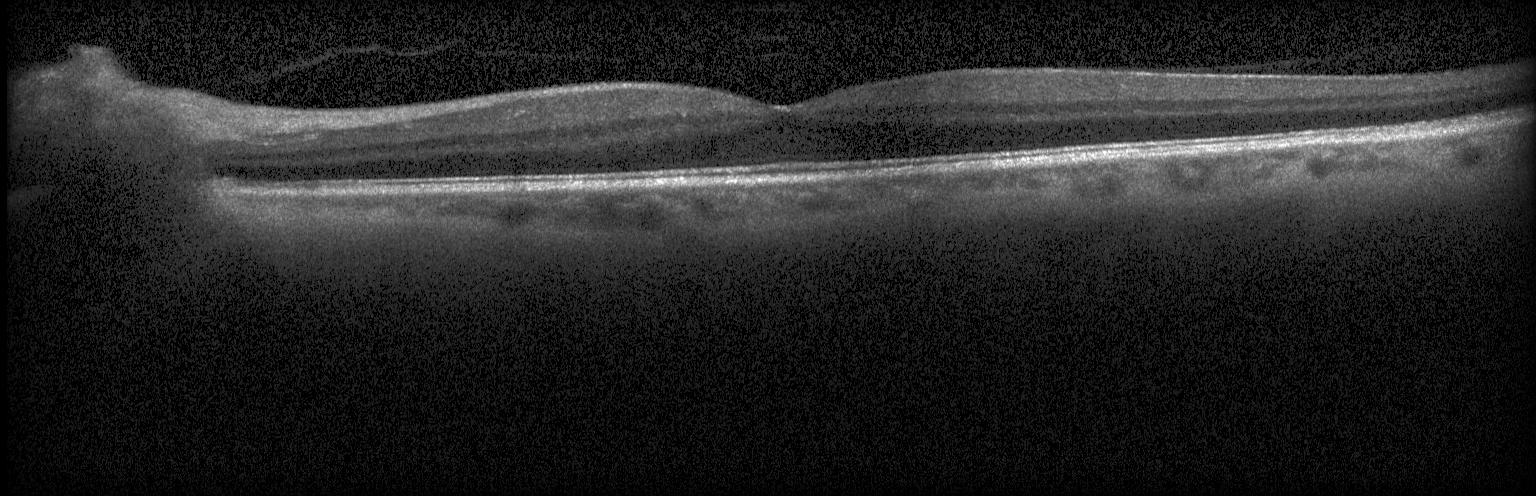
Optical coherence tomography B-scan, spectral-domain OCT, horizontal scan through the fovea, Heidelberg Spectralis OCT system. This B-scan demonstrates no choroidal neovascularization, diabetic macular edema, or drusen.